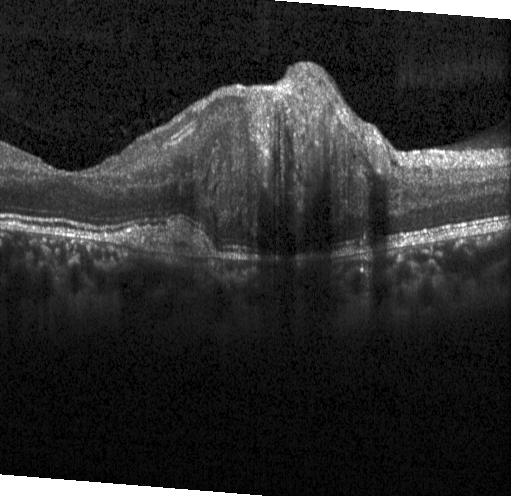

SD-OCT, optical coherence tomography B-scan. Diagnosis: choroidal neovascularization (CNV).